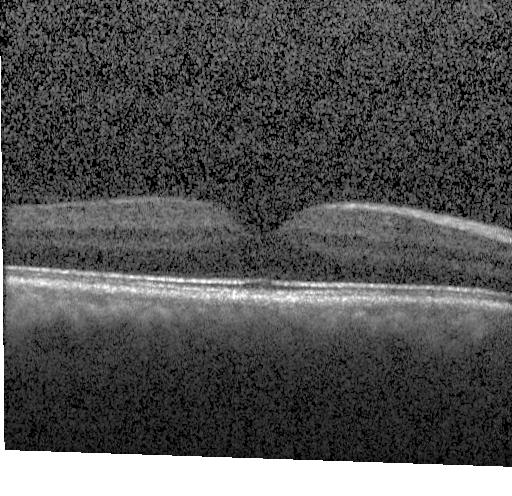
Fovea-centered, OCT line scan, Heidelberg Spectralis, SD-OCT — Dx: neither CNV, DME, nor drusen.